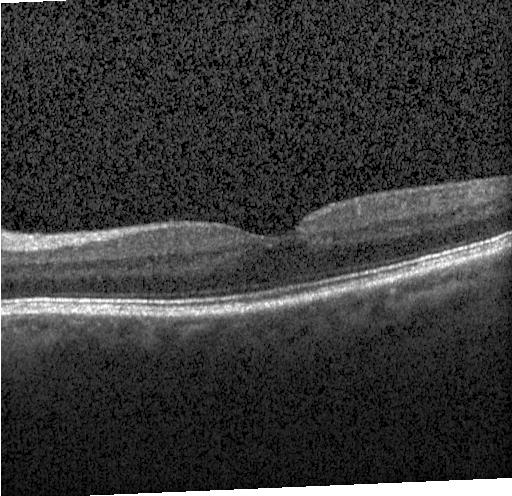 Finding: no evidence of choroidal neovascularization, diabetic macular edema, or drusen.